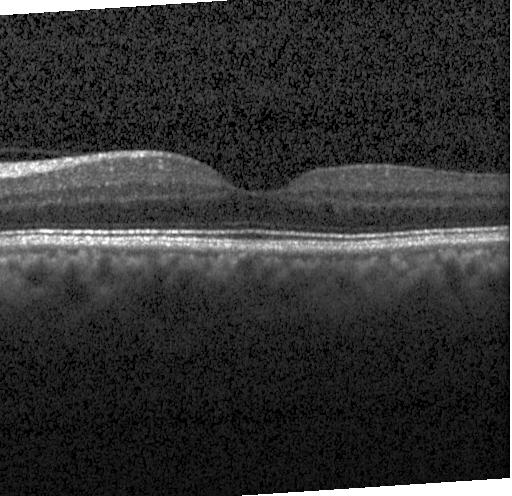

Retinal OCT cross-section. Diagnosis: no choroidal neovascularization, no diabetic macular edema, and no drusen.